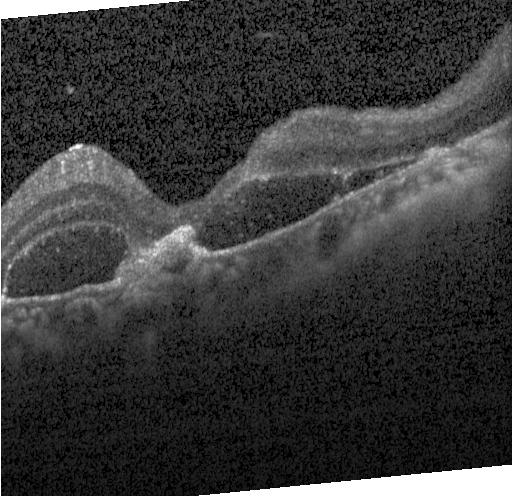 OCT scan showing choroidal neovascularization.